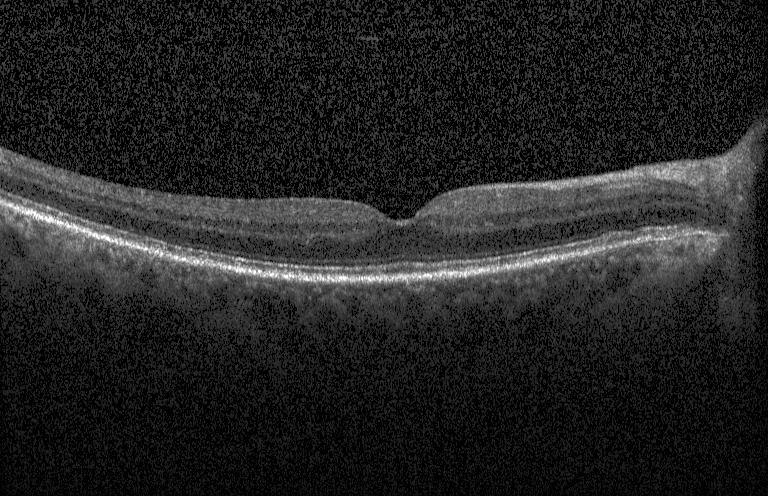
Spectral-domain optical coherence tomography. Heidelberg Spectralis OCT system. Retinal OCT B-scan. Macular scan.
No CNV, no DME, and no drusen.